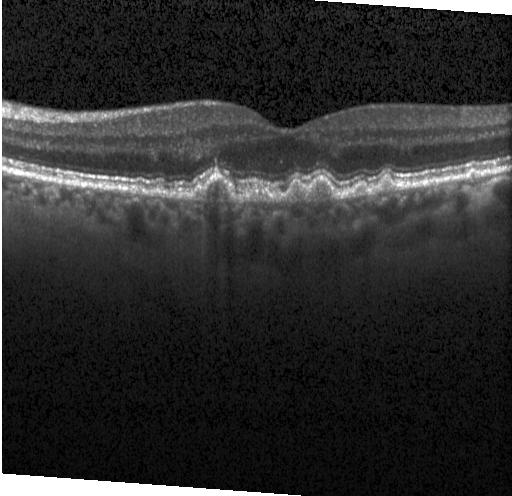 OCT B-scan showing multiple drusen.